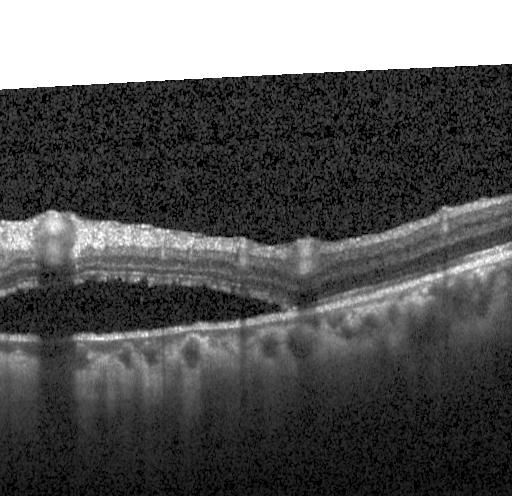 OCT B-scan · spectral-domain OCT · through the macula.
Diagnosis: a choroidal neovascular membrane.